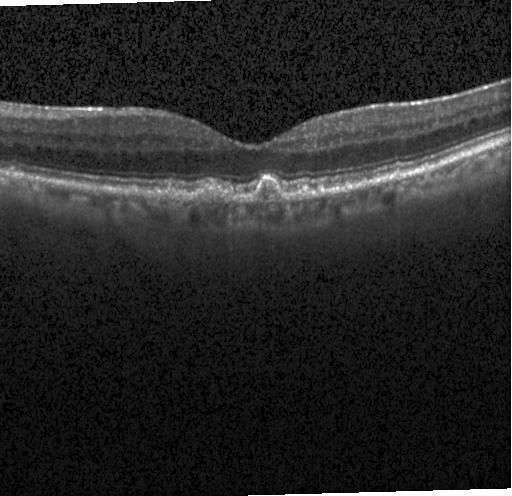 Sub-RPE drusenoid deposits.